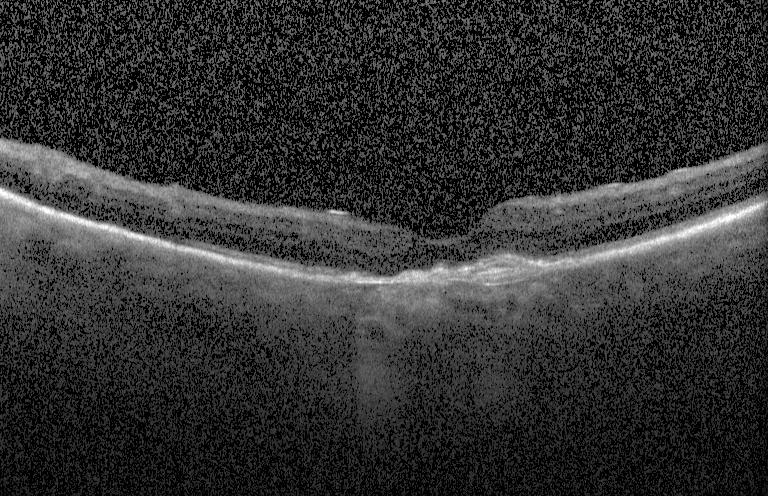
Assessment: a choroidal neovascular membrane.